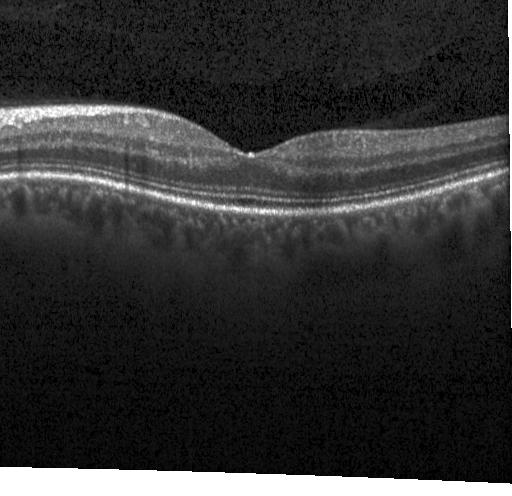
SD-OCT · through the macula · retinal OCT B-scan — Finding: neither CNV, DME, nor drusen.